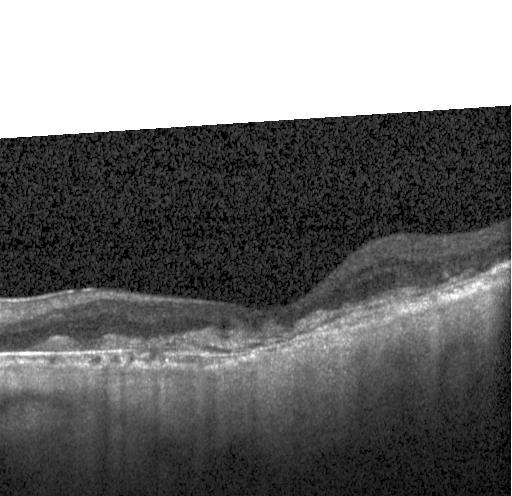 Diagnosis: choroidal neovascularization.